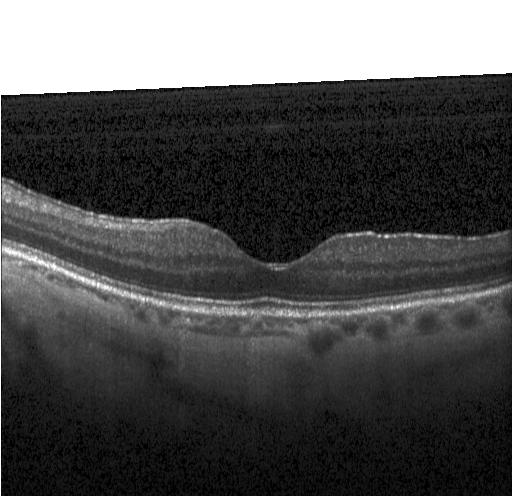
OCT finding: no choroidal neovascularization, no diabetic macular edema, and no drusen.